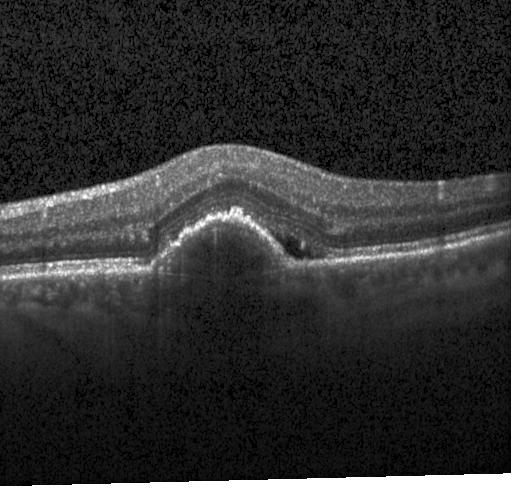

Retinal OCT B-scan. Acquired on a Heidelberg Spectralis. Through the macula. SD-OCT.
Dx: CNV.